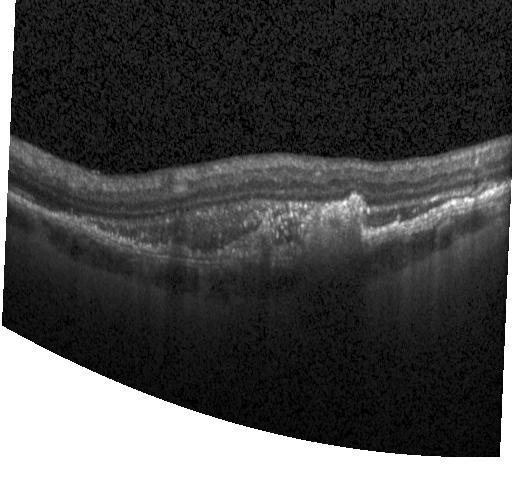

Dx: CNV.